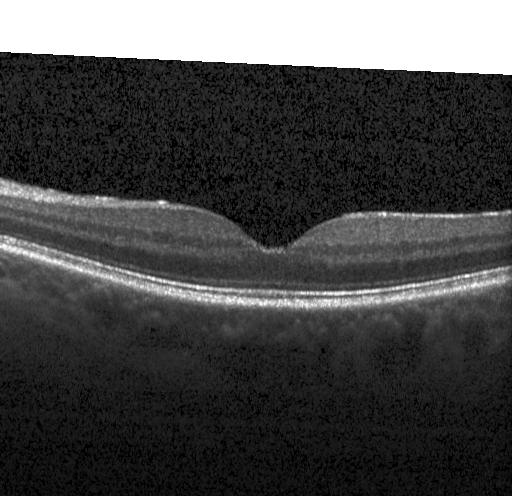

Heidelberg Spectralis; spectral-domain OCT; optical coherence tomography scan; horizontal scan through the fovea.
Impression: no CNV, DME, or drusen.